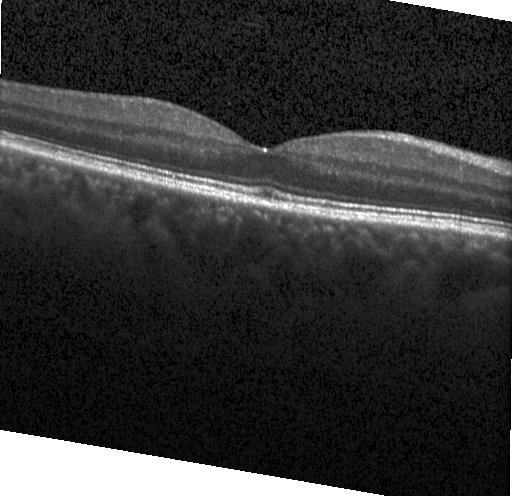

OCT line scan.
Finding: neither choroidal neovascularization, diabetic macular edema, nor drusen.